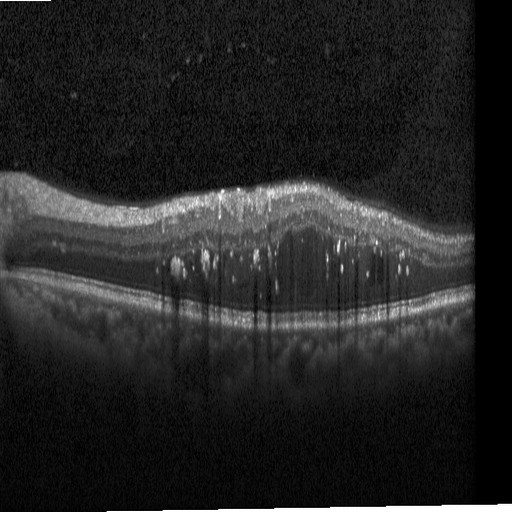 Impression: diabetic macular edema (DME).